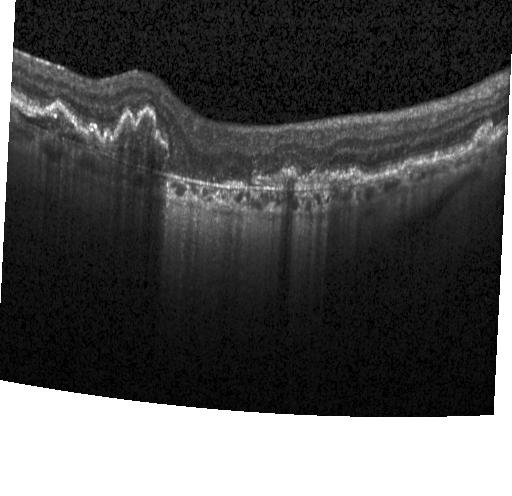
Spectral-domain optical coherence tomography. Optical coherence tomography B-scan. Choroidal neovascularization (CNV).